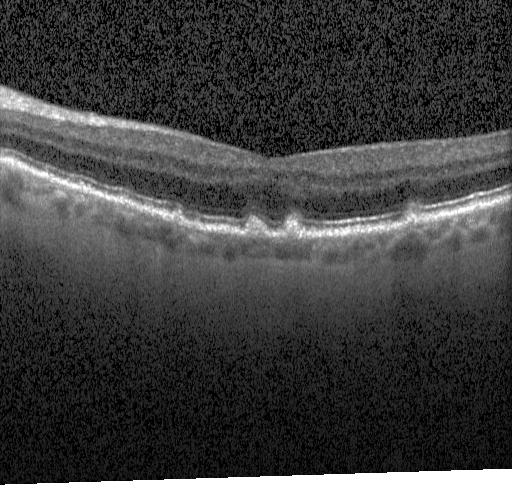

Horizontal scan through the fovea; Heidelberg Spectralis; OCT B-scan; SD-OCT. OCT finding: multiple drusen.